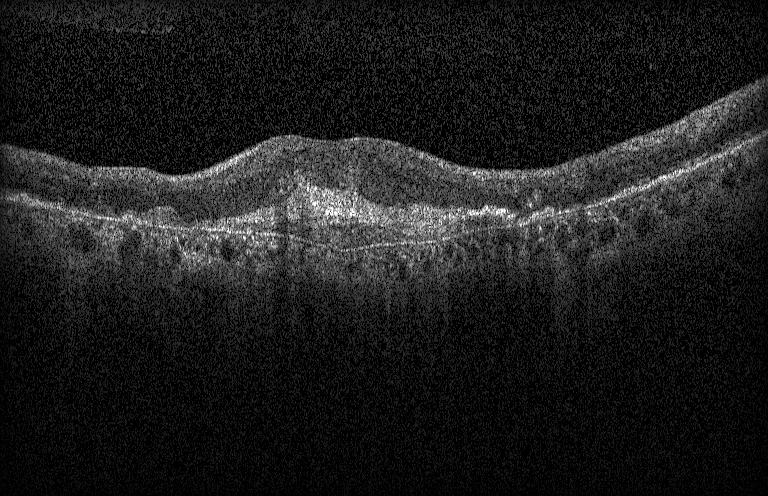
Optical coherence tomography B-scan. Heidelberg Spectralis OCT system.
Macular OCT: a choroidal neovascular membrane.